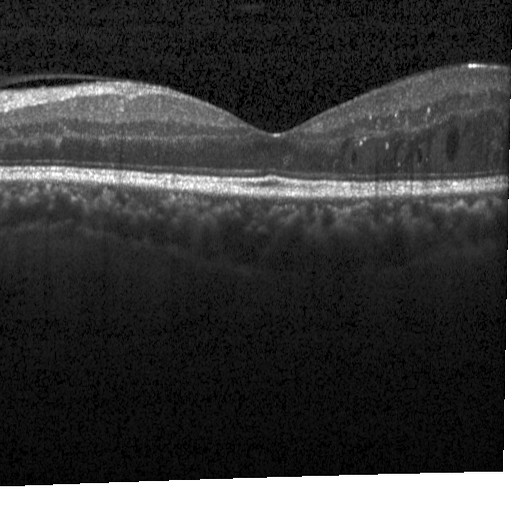

OCT B-scan. Dx: DME.